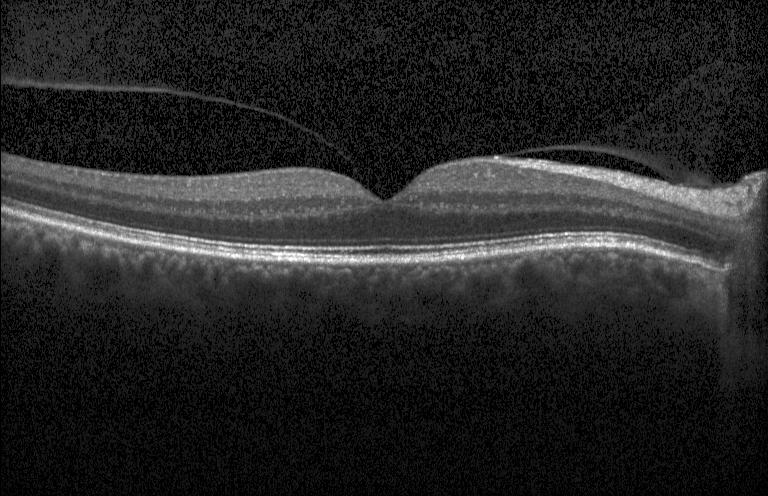
Finding: neither choroidal neovascularization, diabetic macular edema, nor drusen.